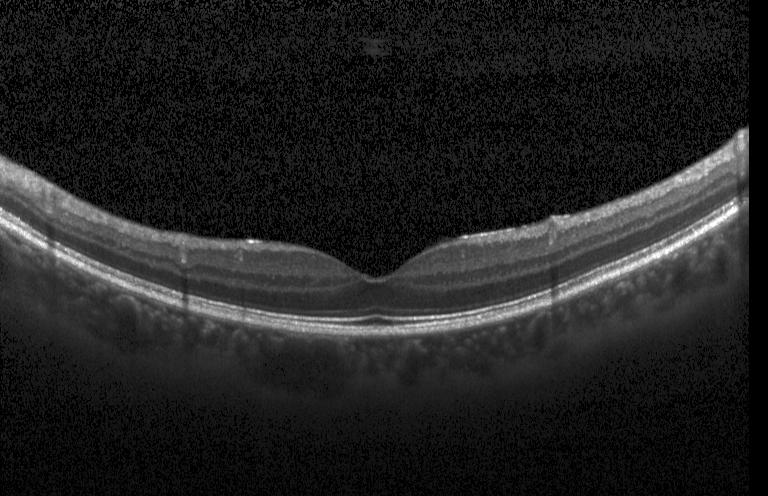 Impression: neither choroidal neovascularization, diabetic macular edema, nor drusen.